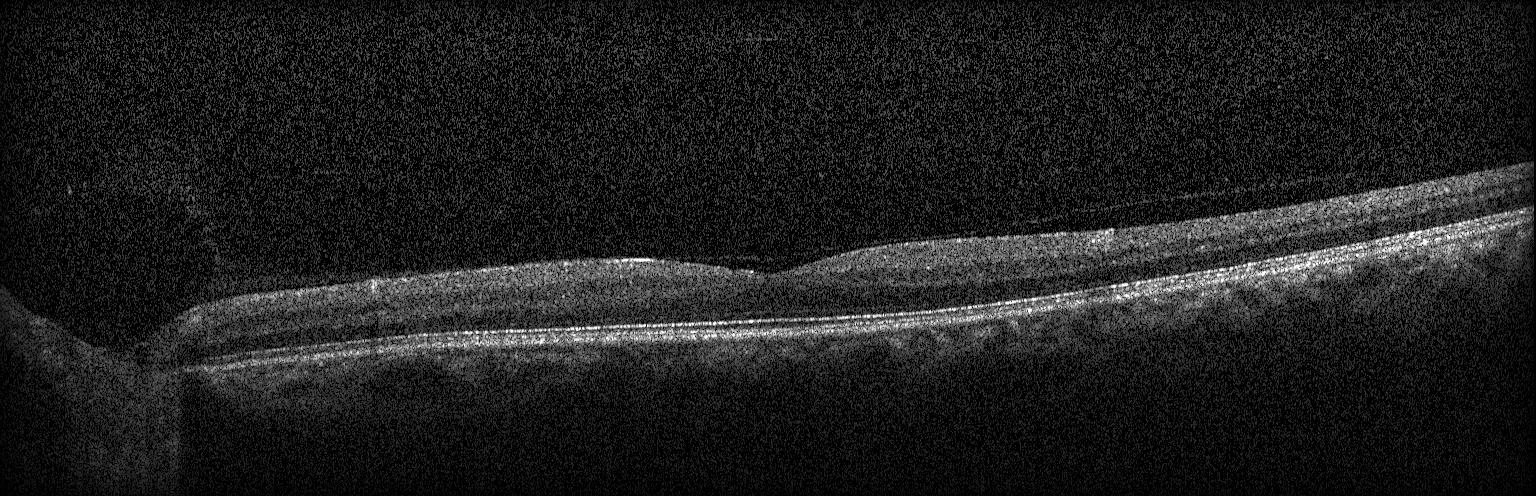

Heidelberg Spectralis OCT system. Through the macula. Optical coherence tomography scan
Impression: no choroidal neovascularization, diabetic macular edema, or drusen.